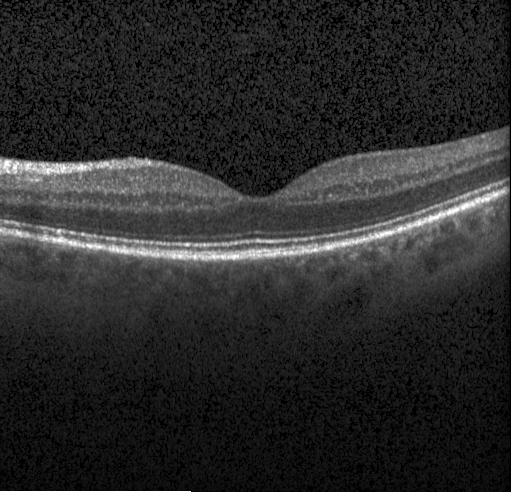
Centered on the fovea, optical coherence tomography B-scan — Finding: neither choroidal neovascularization, diabetic macular edema, nor drusen.